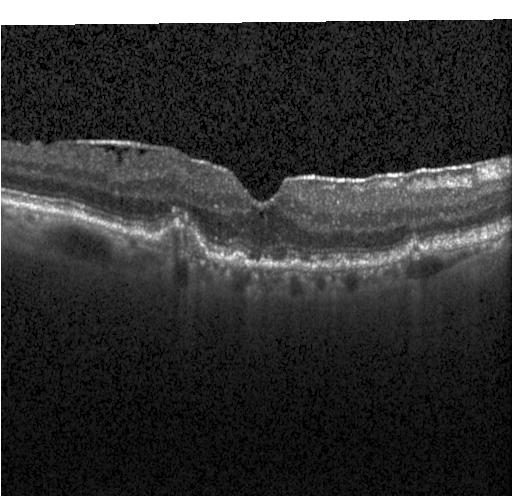
The scan shows sub-RPE drusenoid deposits.